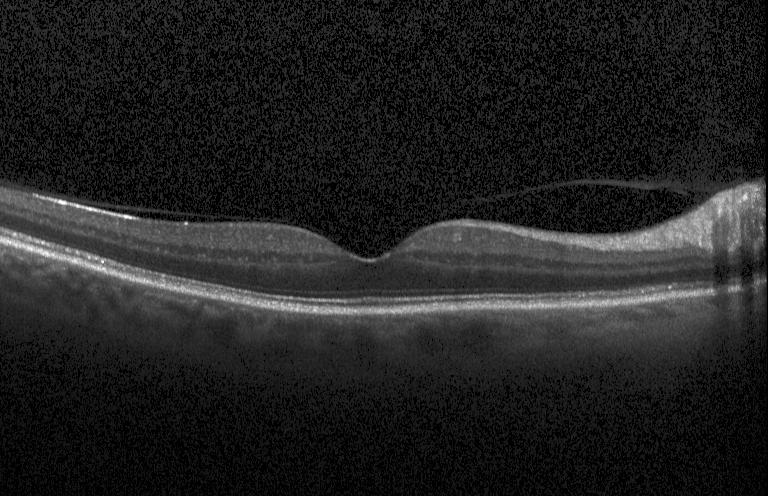 OCT B-scan showing no CNV, DME, or drusen.